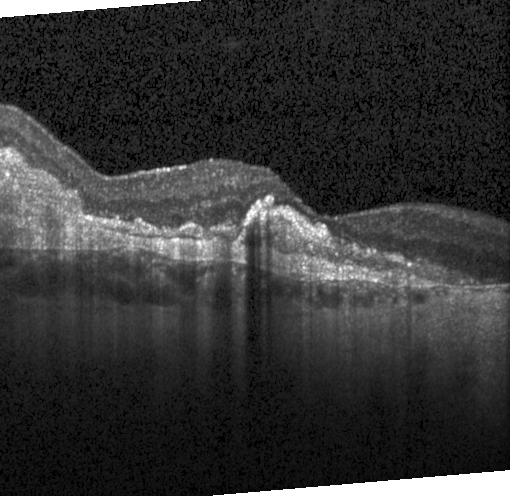
Macular OCT demonstrating CNV.